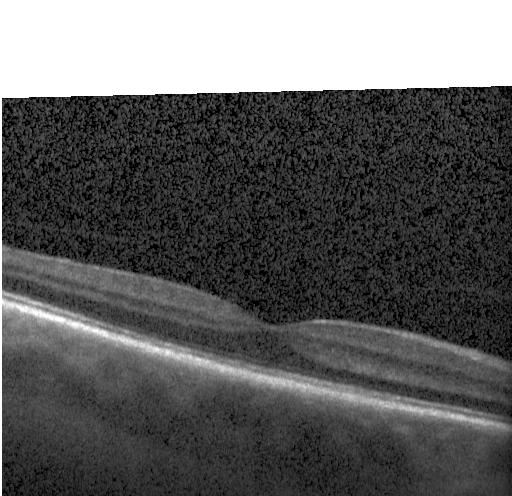 Spectral-domain OCT; retinal OCT B-scan
Macular OCT: no choroidal neovascularization, diabetic macular edema, or drusen.